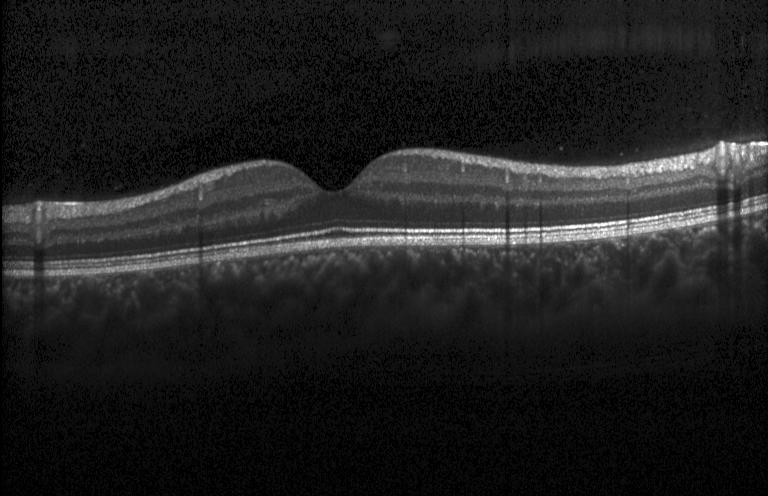 Retinal OCT cross-section · spectral-domain OCT. OCT finding: no choroidal neovascularization, no diabetic macular edema, and no drusen.